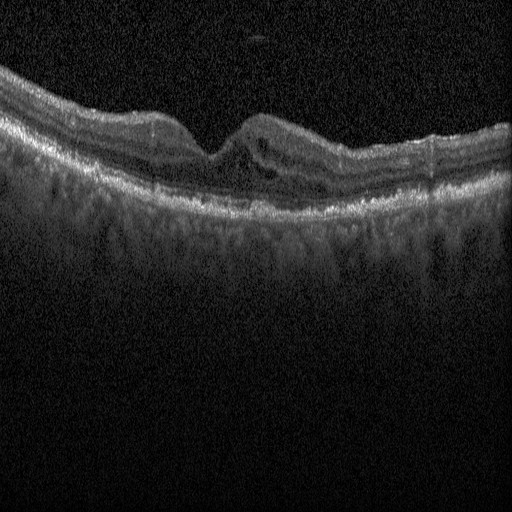 OCT B-scan.
Impression: diabetic macular edema (DME).